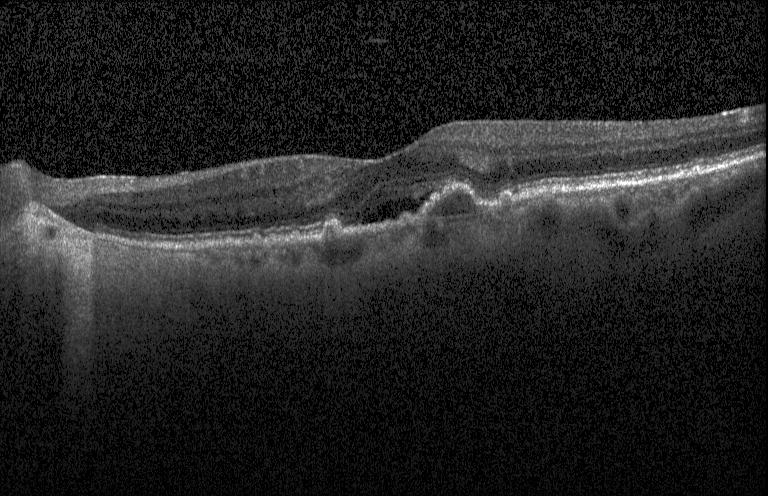 Macular OCT: choroidal neovascularization.